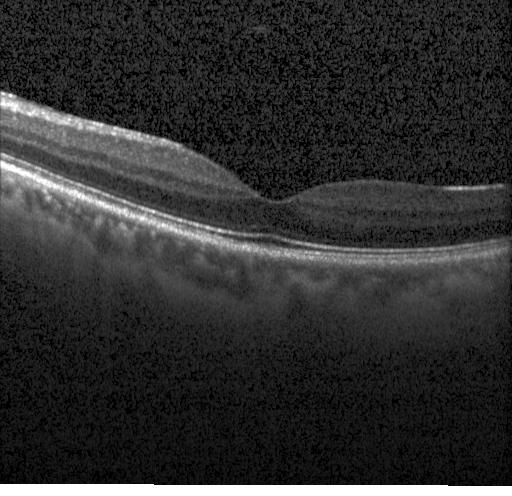
Diagnosis: no evidence of choroidal neovascularization, diabetic macular edema, or drusen.